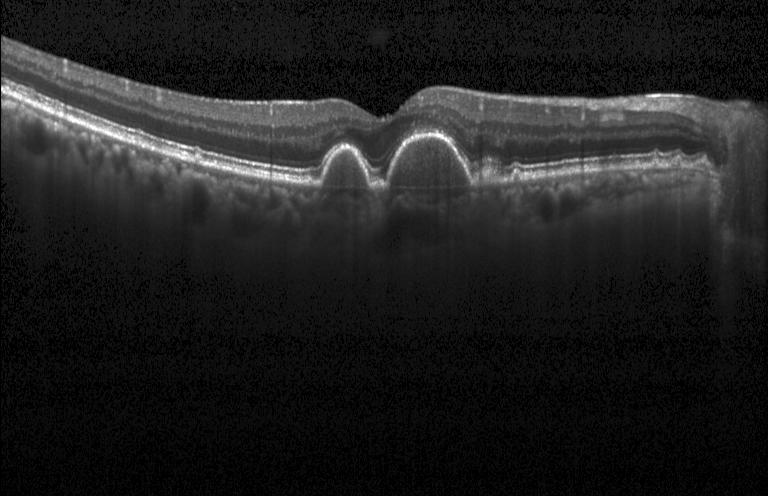

OCT scan showing drusen.